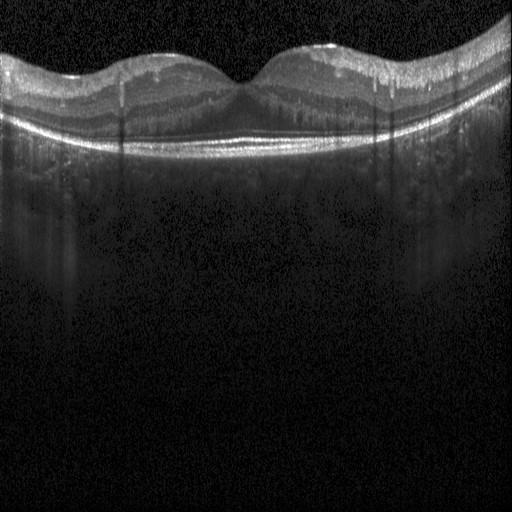

Centered on the fovea; optical coherence tomography B-scan; acquired on a Heidelberg Spectralis. The scan shows DME.